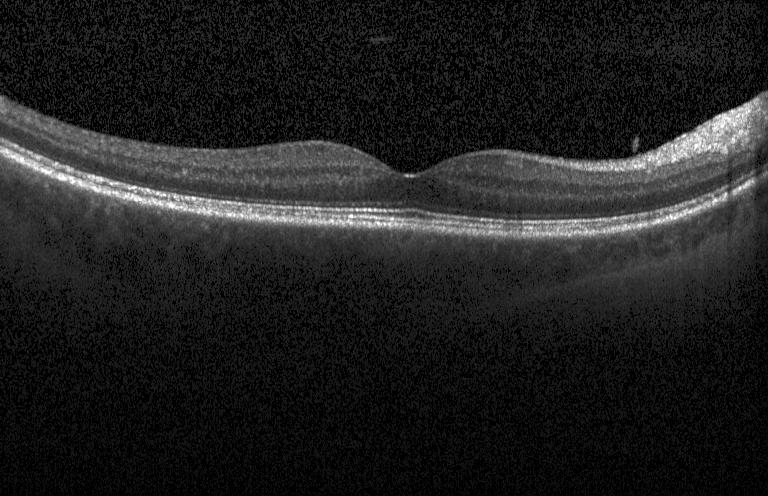

Diagnosis: no CNV, DME, or drusen.